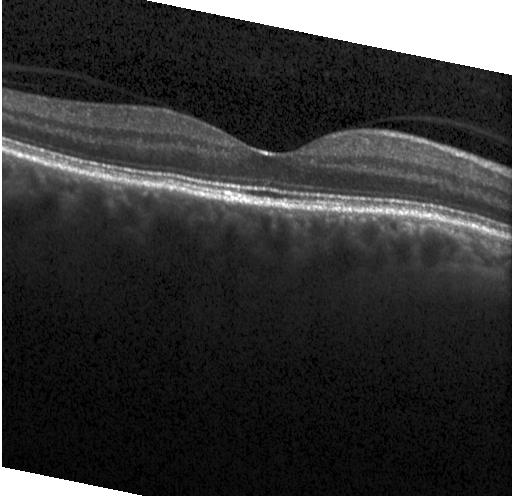

Spectral-domain optical coherence tomography, macular scan, OCT line scan — Impression: no choroidal neovascularization, no diabetic macular edema, and no drusen.